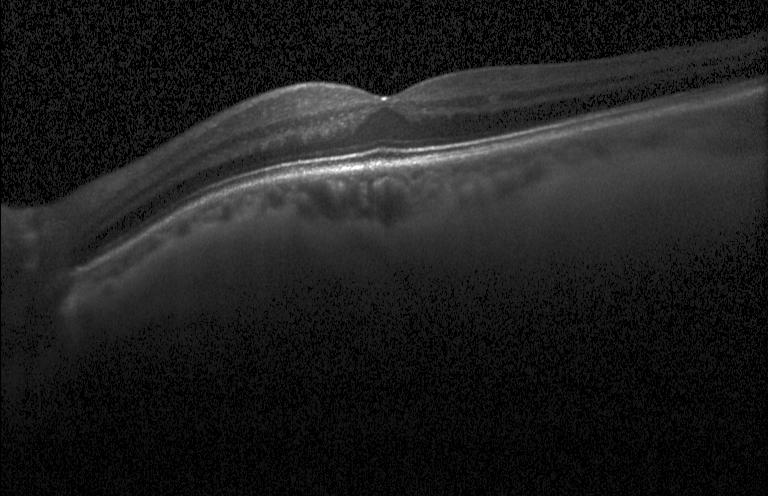

Finding: neither choroidal neovascularization, diabetic macular edema, nor drusen.